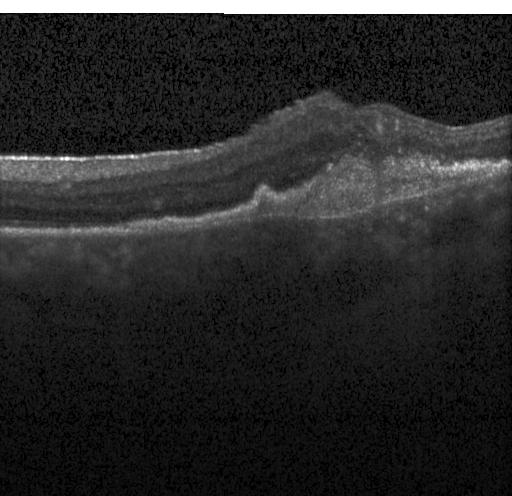 Diagnosis: choroidal neovascularization.